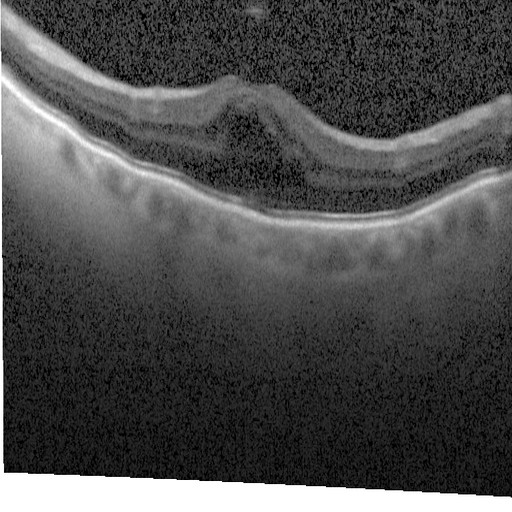 OCT finding: DME.